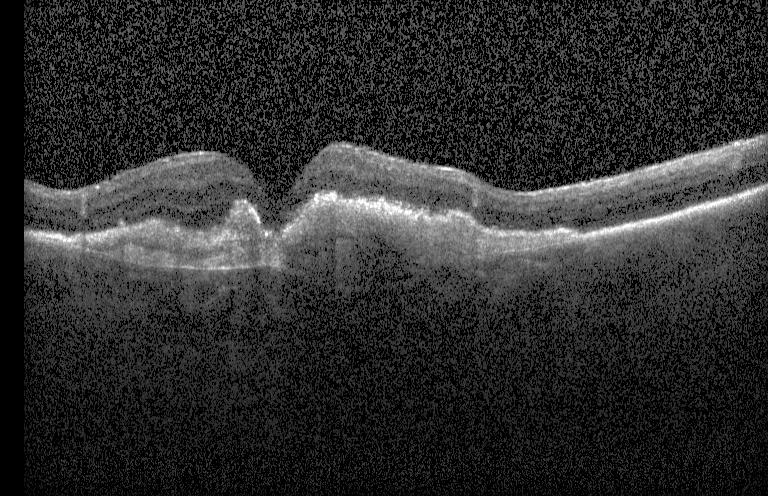

OCT B-scan. Fovea-centered. Acquired on a Heidelberg Spectralis
This B-scan demonstrates choroidal neovascularization (CNV).